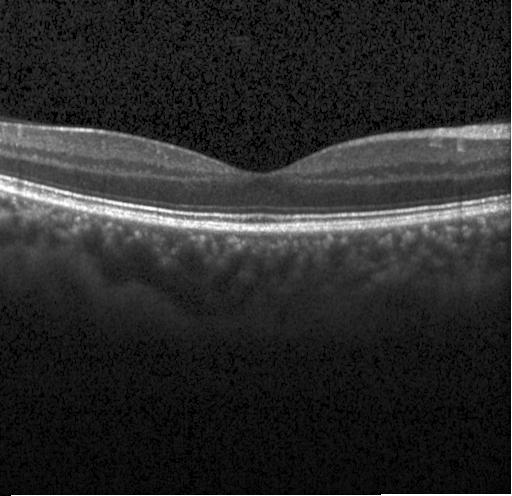 Macular OCT: no choroidal neovascularization, no diabetic macular edema, and no drusen.